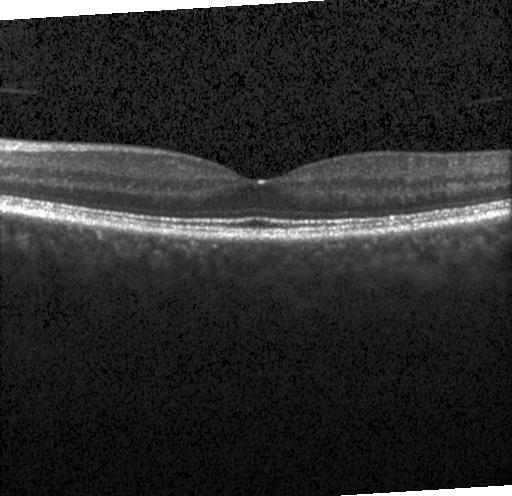

OCT scan showing no evidence of choroidal neovascularization, diabetic macular edema, or drusen.